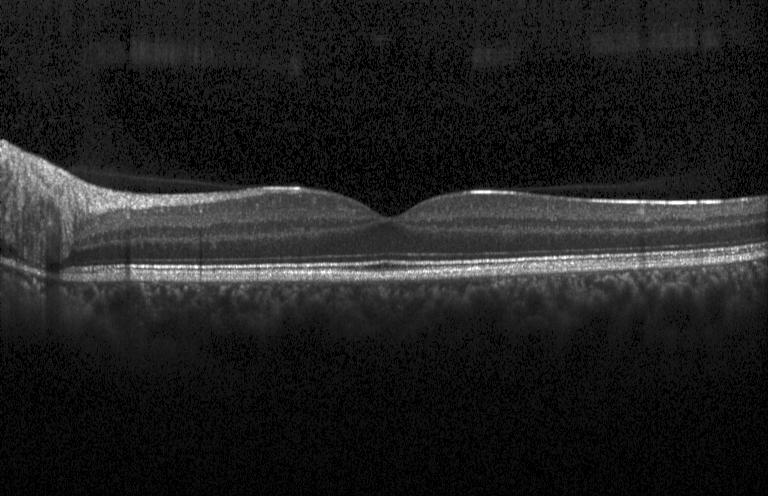 Instrument: Heidelberg Spectralis, spectral-domain OCT, through the macula, OCT B-scan.
No CNV, DME, or drusen.